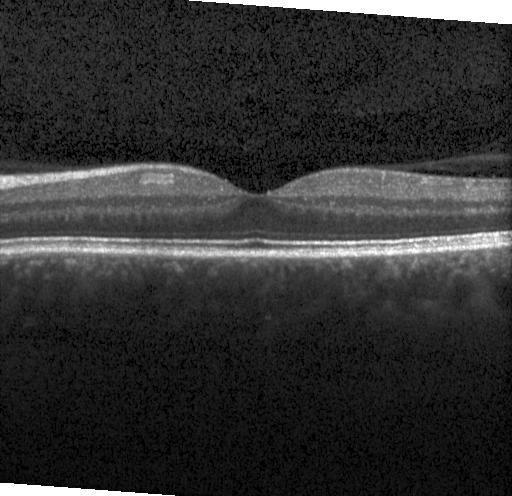

Spectral-domain optical coherence tomography; optical coherence tomography scan; through the macula. Finding: no choroidal neovascularization, no diabetic macular edema, and no drusen.